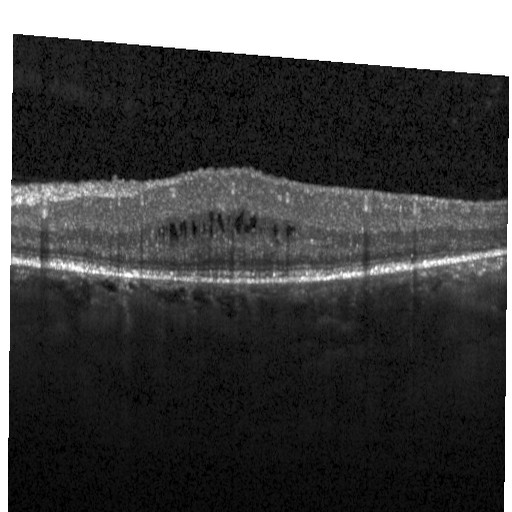

Optical coherence tomography B-scan · spectral-domain optical coherence tomography · Heidelberg Spectralis OCT system · centered on the fovea.
DME.